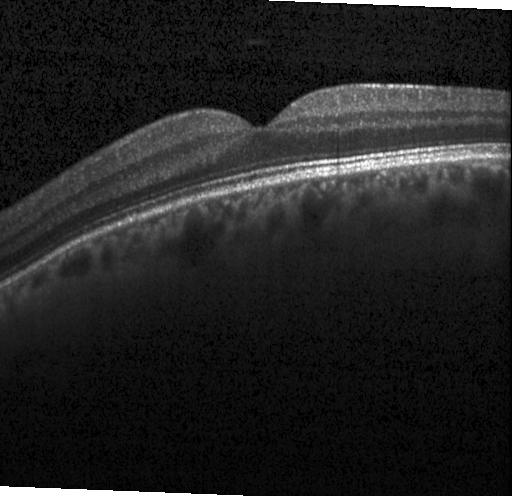 OCT scan showing neither choroidal neovascularization, diabetic macular edema, nor drusen.